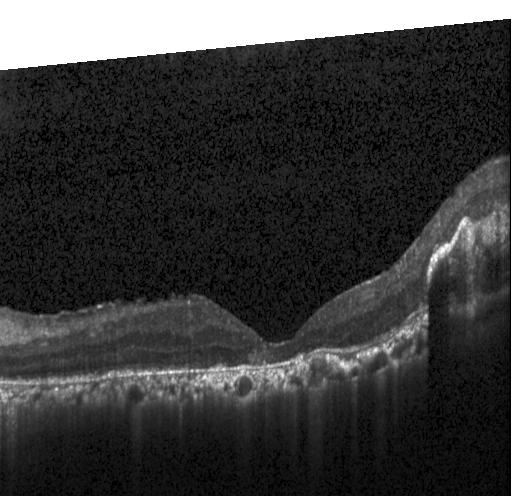 Optical coherence tomography B-scan
This B-scan demonstrates choroidal neovascularization (CNV).